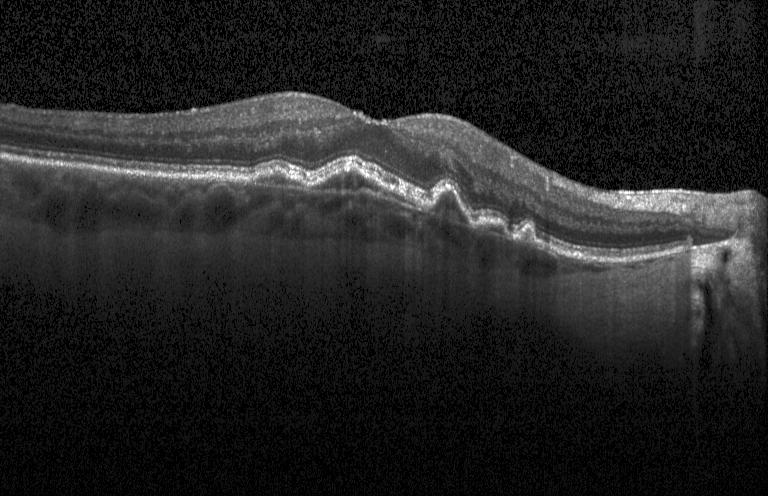

Finding: CNV.